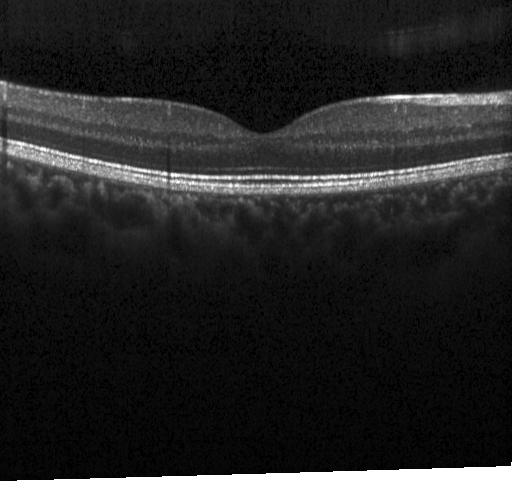 The scan shows no evidence of CNV, DME, or drusen.